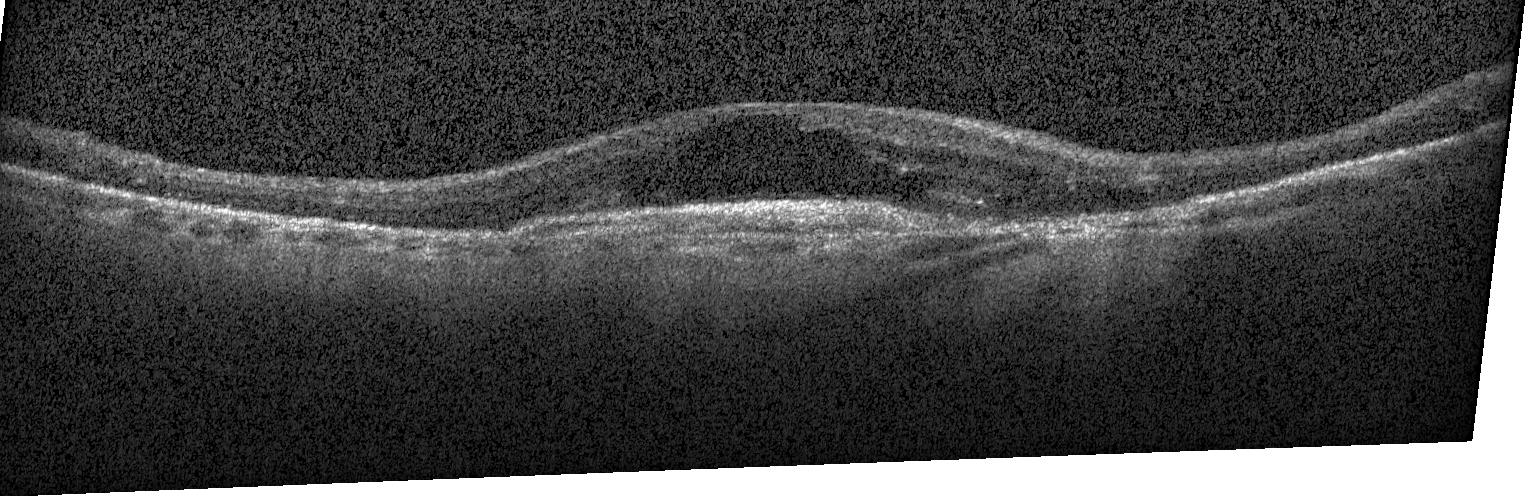

Acquired on a Heidelberg Spectralis · OCT line scan
Impression: choroidal neovascularization.